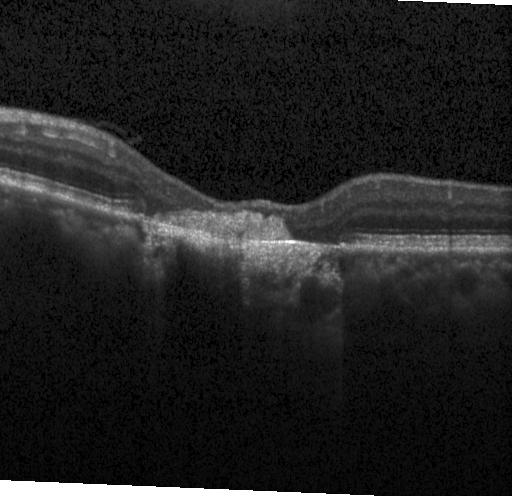 Horizontal scan through the fovea, retinal OCT cross-section, spectral-domain optical coherence tomography, Heidelberg Spectralis.
Assessment: a choroidal neovascular membrane.